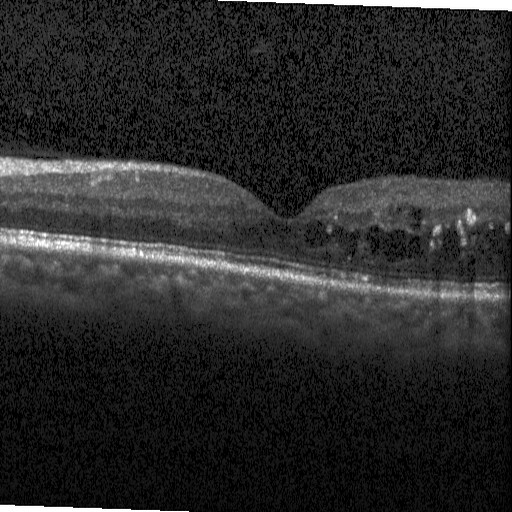

Dx: diabetic macular edema (DME).